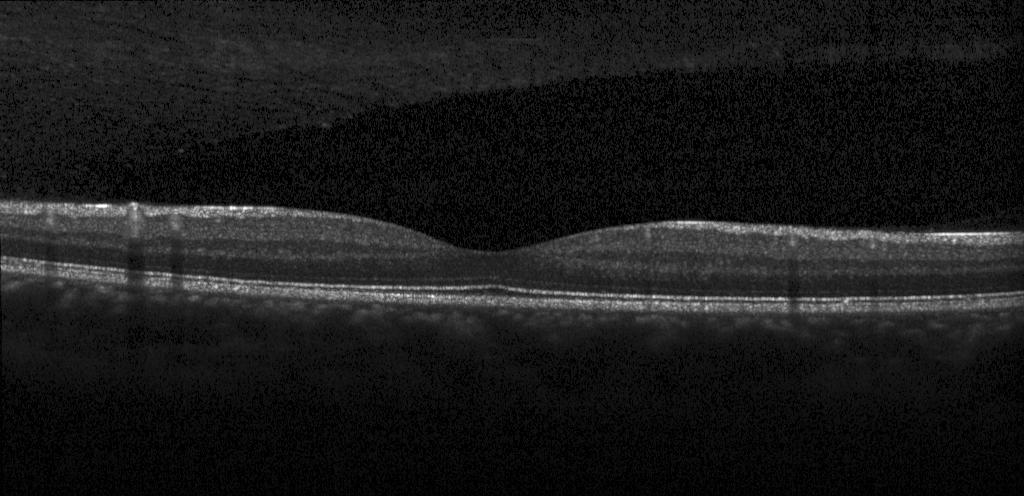

Heidelberg Spectralis OCT system; OCT line scan
Finding: no evidence of choroidal neovascularization, diabetic macular edema, or drusen.